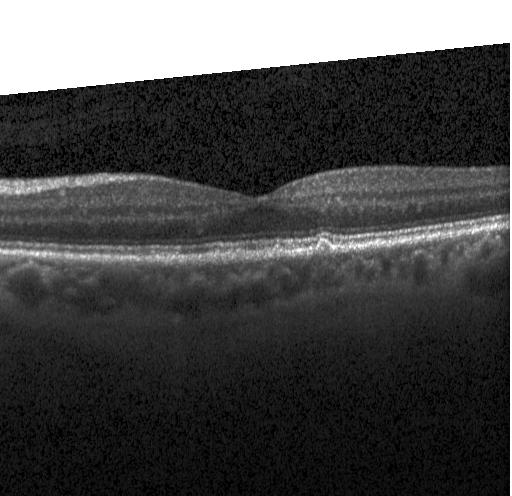
Finding: drusen.